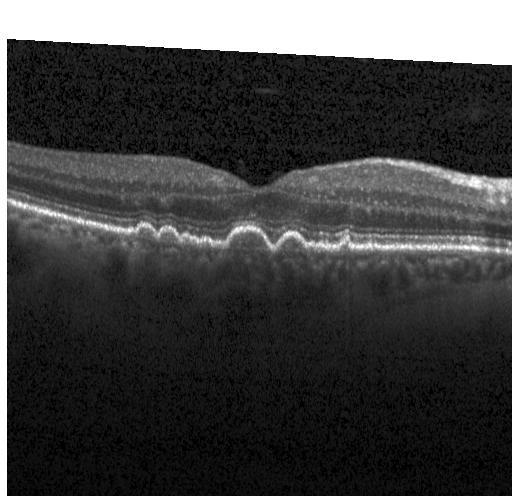 Retinal OCT B-scan
Diagnosis: sub-RPE drusenoid deposits.